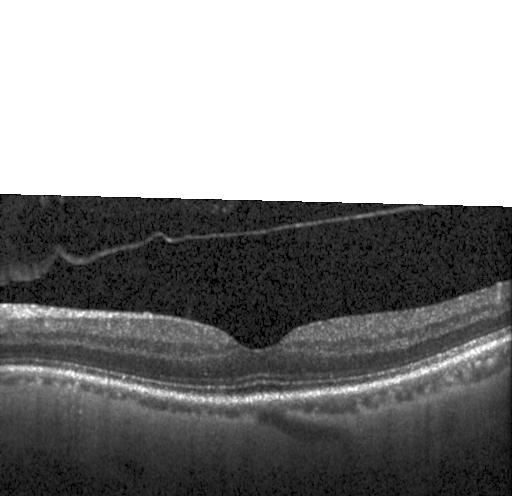 Centered on the fovea, acquired on a Heidelberg Spectralis, OCT B-scan. Impression: neither CNV, DME, nor drusen.